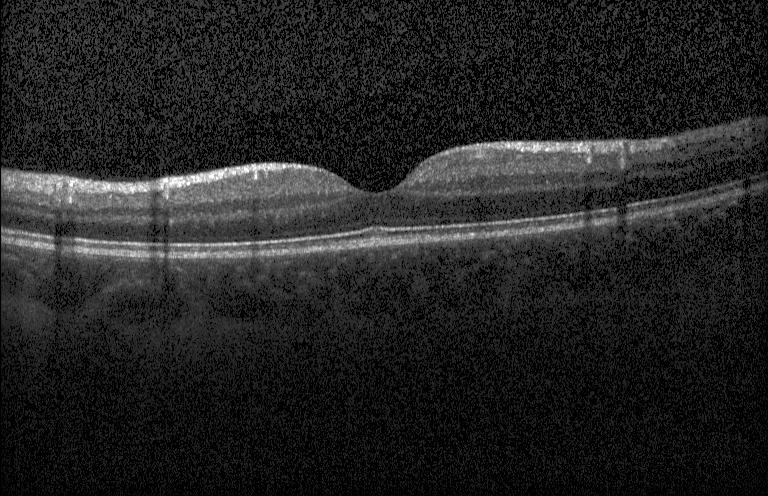

Impression: no choroidal neovascularization, diabetic macular edema, or drusen.